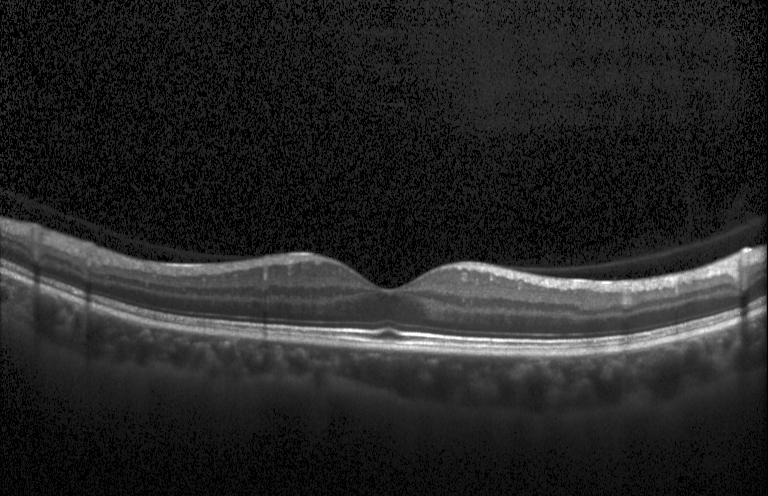 Retinal OCT cross-section showing no evidence of choroidal neovascularization, diabetic macular edema, or drusen.